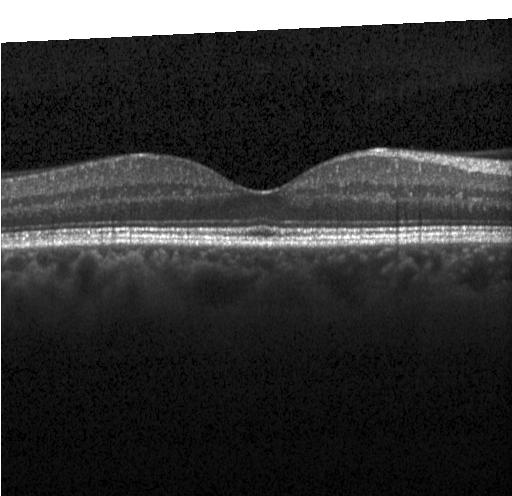

Retinal OCT cross-section; acquired on a Heidelberg Spectralis.
Dx: neither choroidal neovascularization, diabetic macular edema, nor drusen.